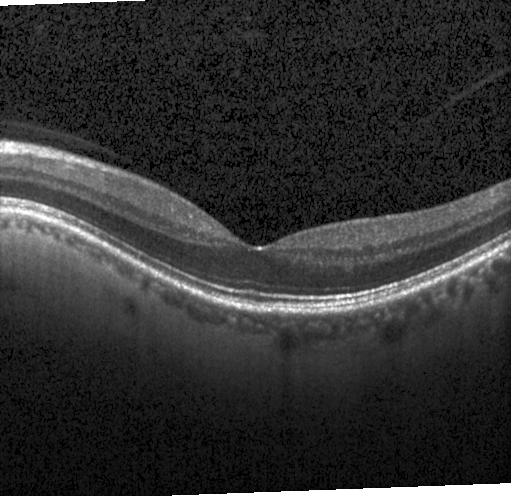 Fovea-centered. Heidelberg Spectralis OCT system. Spectral-domain optical coherence tomography. Retinal OCT B-scan.
Macular OCT: no choroidal neovascularization, diabetic macular edema, or drusen.